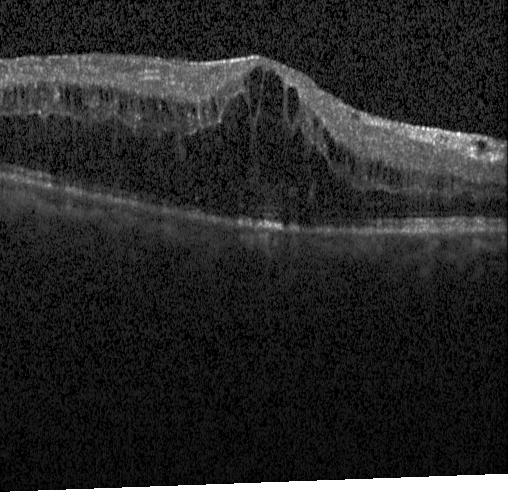

Finding: diabetic macular edema (DME).